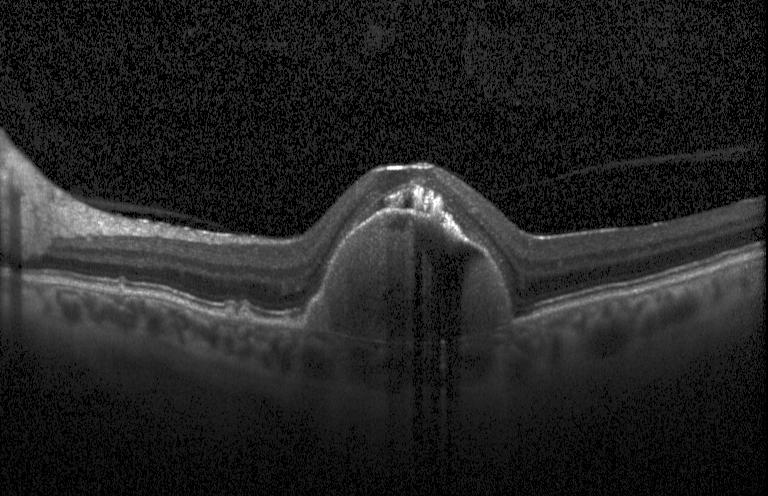

Retinal OCT B-scan
Impression: a choroidal neovascular membrane.